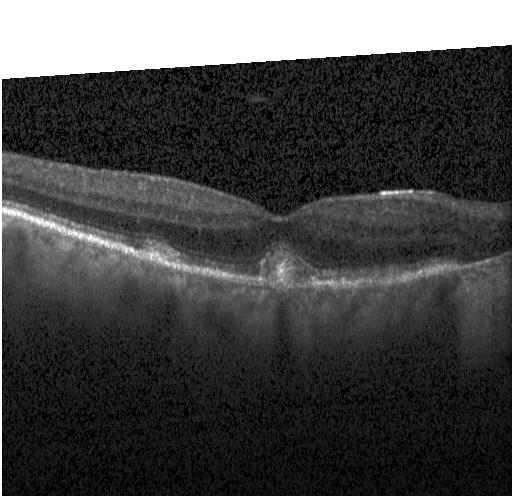 OCT scan showing choroidal neovascularization.